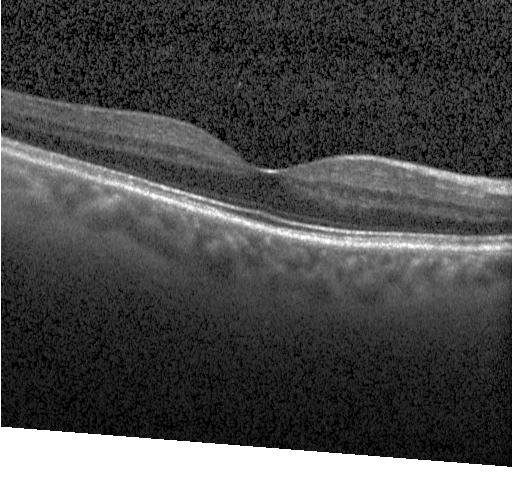 Macular OCT demonstrating no choroidal neovascularization, no diabetic macular edema, and no drusen.